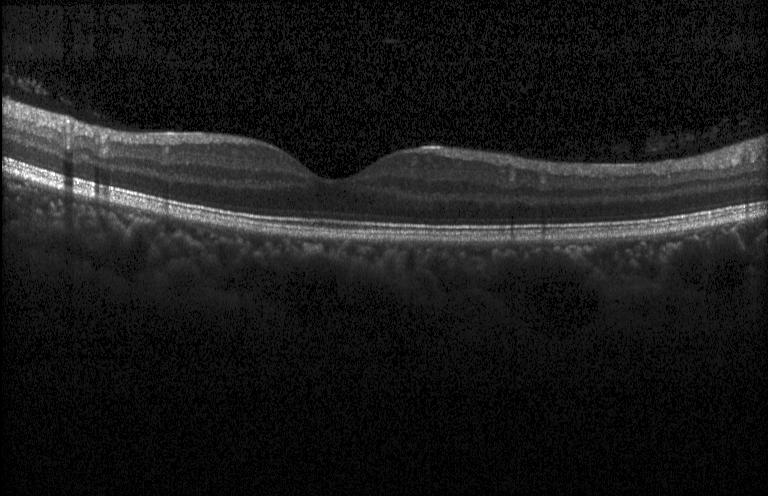

Neither choroidal neovascularization, diabetic macular edema, nor drusen.